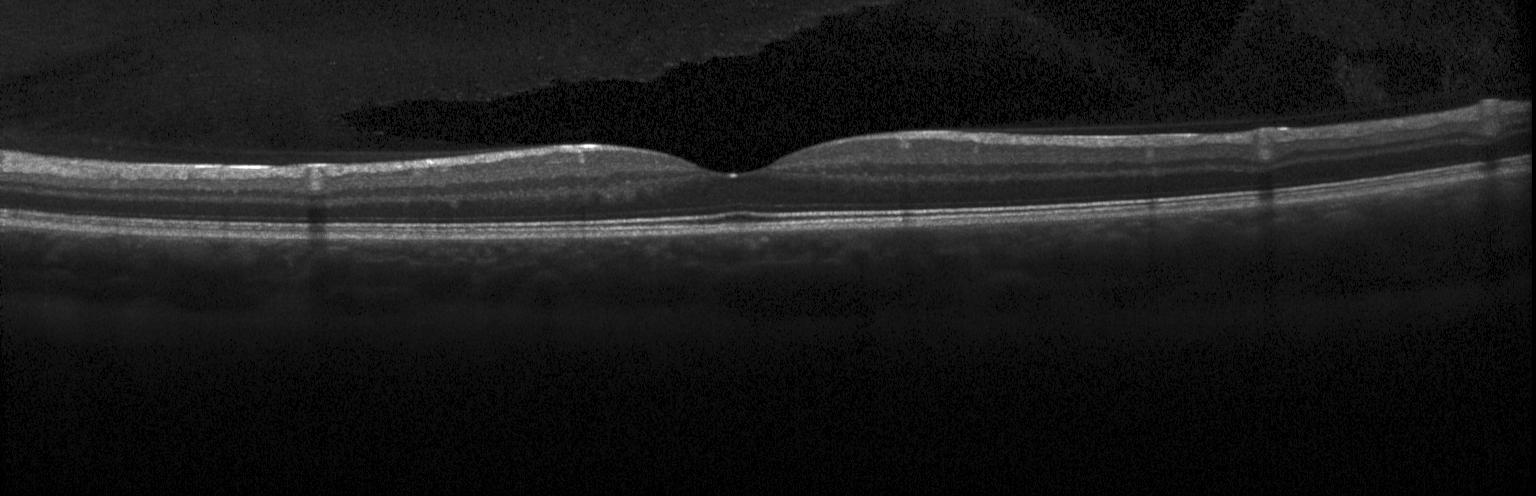

Through the macula. SD-OCT. Retinal OCT cross-section. Heidelberg Spectralis OCT system
Impression: no evidence of choroidal neovascularization, diabetic macular edema, or drusen.